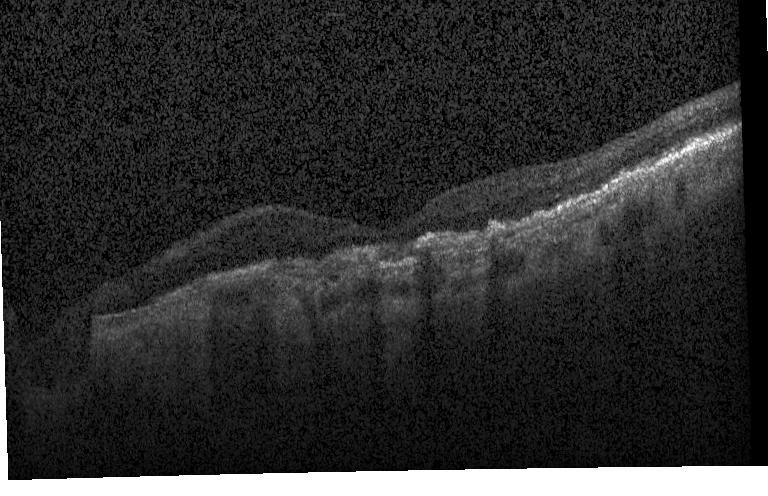

Heidelberg Spectralis; spectral-domain optical coherence tomography; OCT B-scan; macular scan. Diagnosis: a choroidal neovascular membrane.